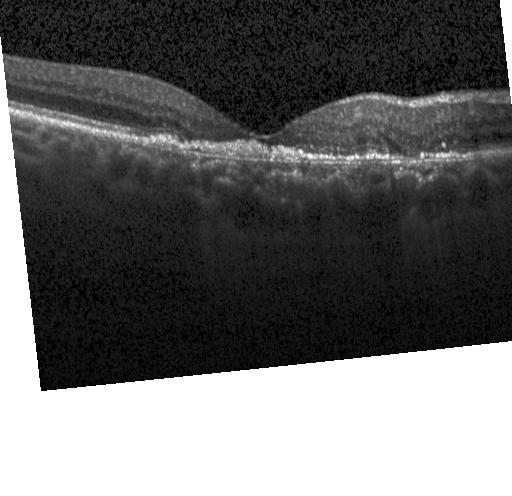 Diagnosis: a choroidal neovascular membrane.